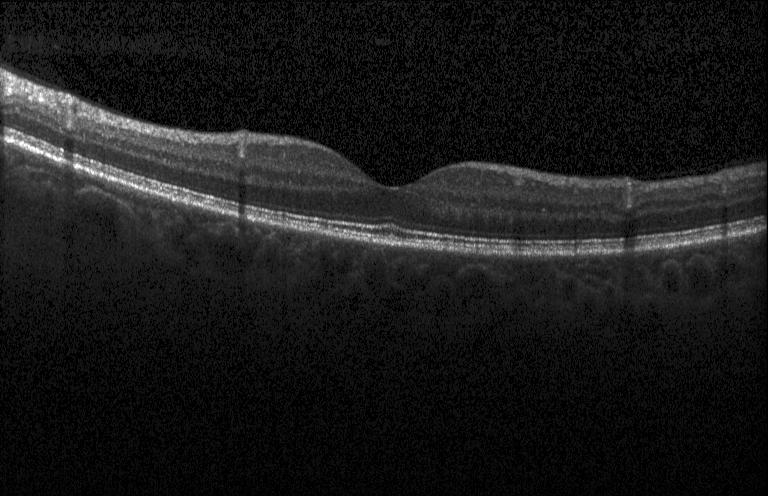 Fovea-centered. SD-OCT. Instrument: Heidelberg Spectralis. OCT line scan
Diagnosis: no evidence of CNV, DME, or drusen.